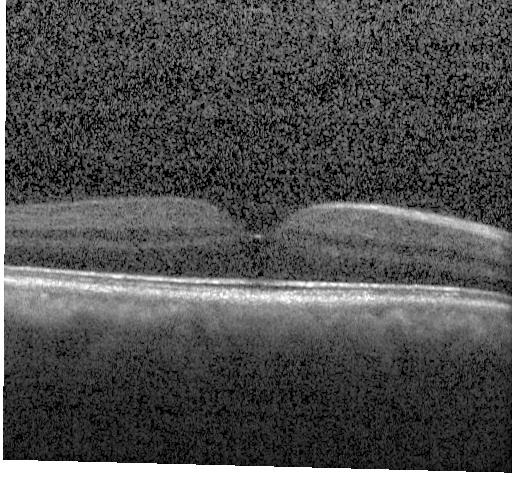 SD-OCT · Heidelberg Spectralis OCT system · through the macula · optical coherence tomography scan — Diagnosis: neither choroidal neovascularization, diabetic macular edema, nor drusen.